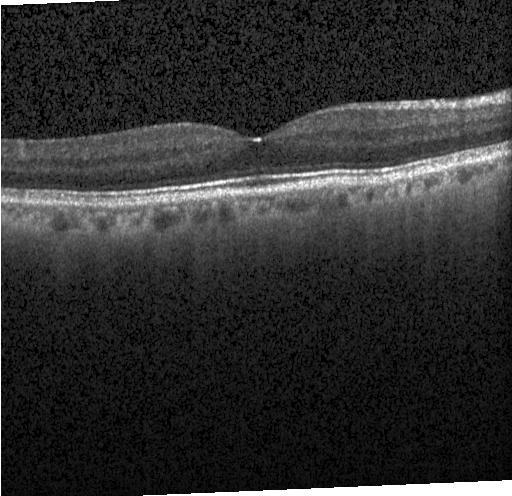

Assessment: no evidence of CNV, DME, or drusen.